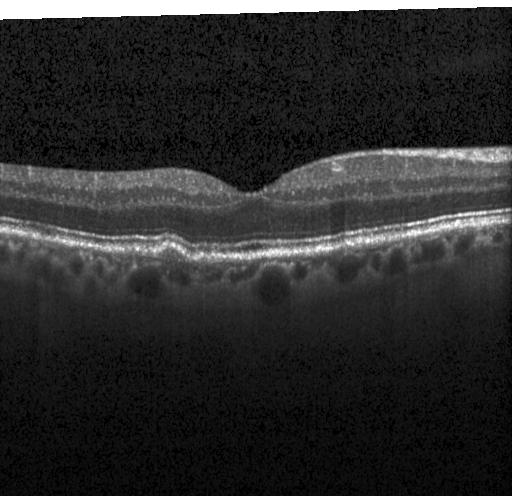
Centered on the fovea, optical coherence tomography B-scan, instrument: Heidelberg Spectralis, spectral-domain OCT
Finding: drusen.